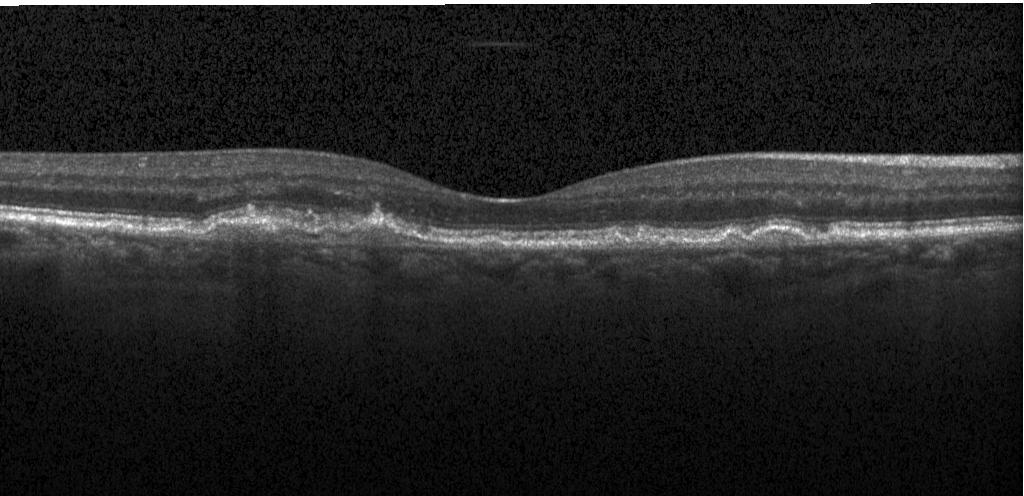 Through the macula; Heidelberg Spectralis OCT system; optical coherence tomography scan
The scan shows choroidal neovascularization (CNV).